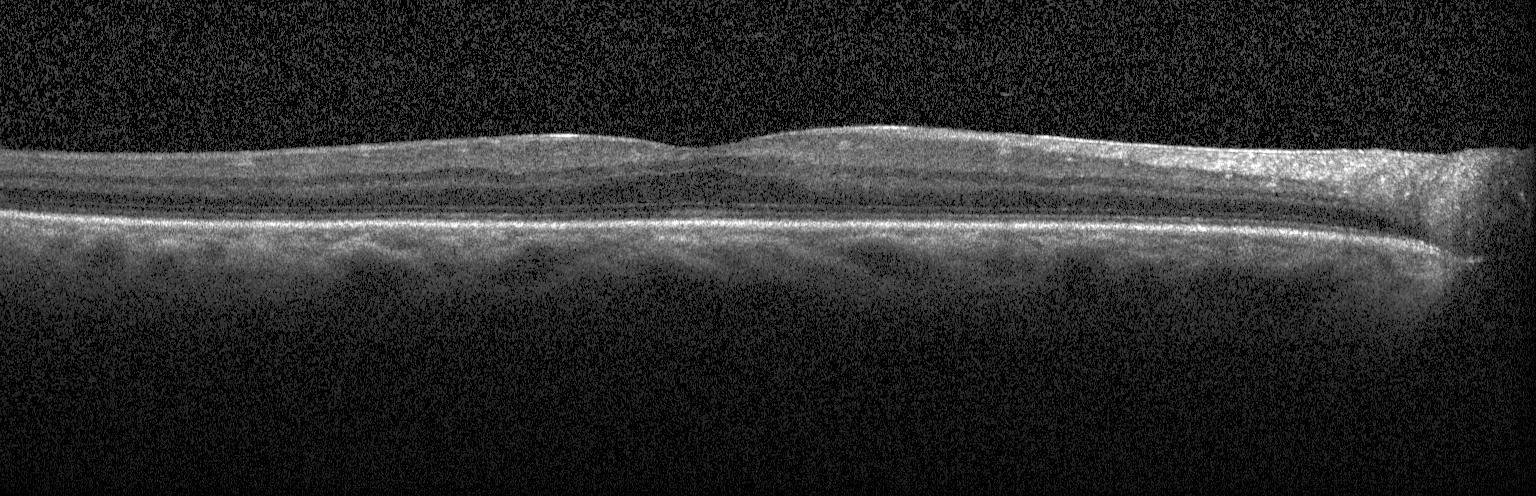
Instrument: Heidelberg Spectralis, optical coherence tomography B-scan
OCT finding: neither choroidal neovascularization, diabetic macular edema, nor drusen.